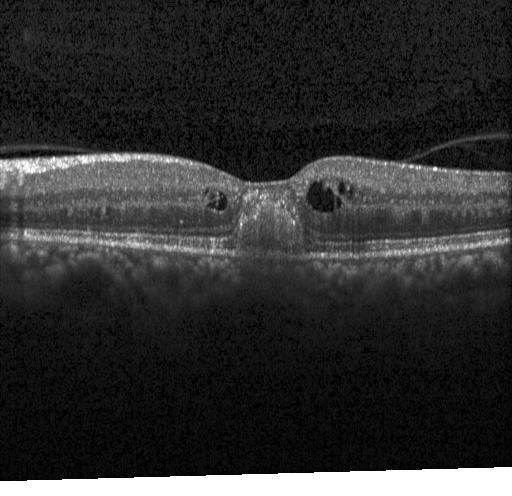

OCT B-scan; centered on the fovea. Diagnosis: choroidal neovascularization.